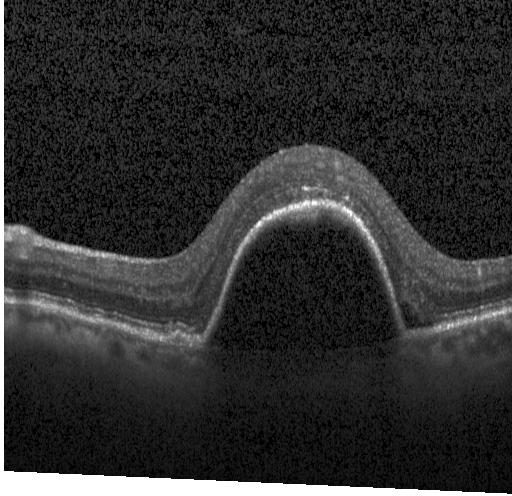
Optical coherence tomography scan · spectral-domain optical coherence tomography · Heidelberg Spectralis OCT system.
Finding: choroidal neovascularization (CNV).